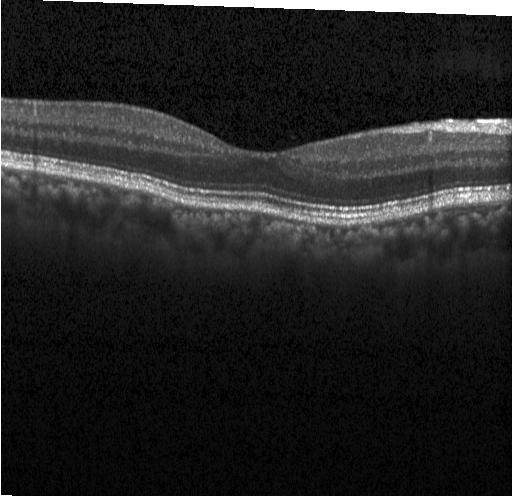 The scan shows no evidence of choroidal neovascularization, diabetic macular edema, or drusen.